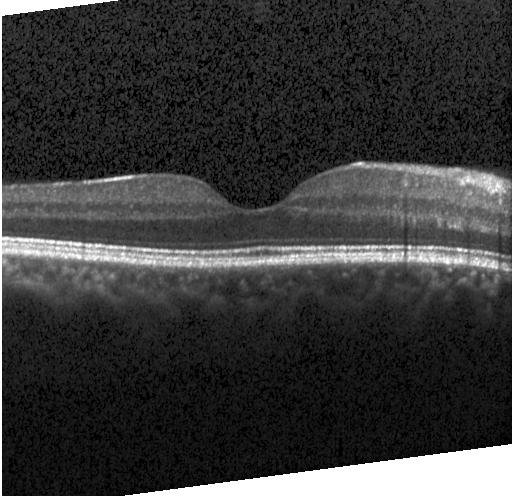
Finding: neither choroidal neovascularization, diabetic macular edema, nor drusen.